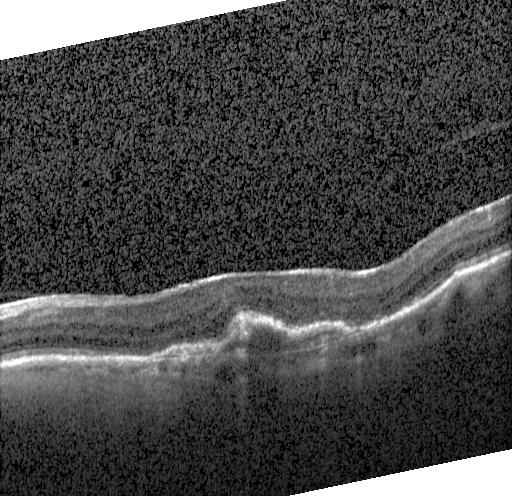 Spectral-domain optical coherence tomography; optical coherence tomography scan
The scan shows choroidal neovascularization (CNV).